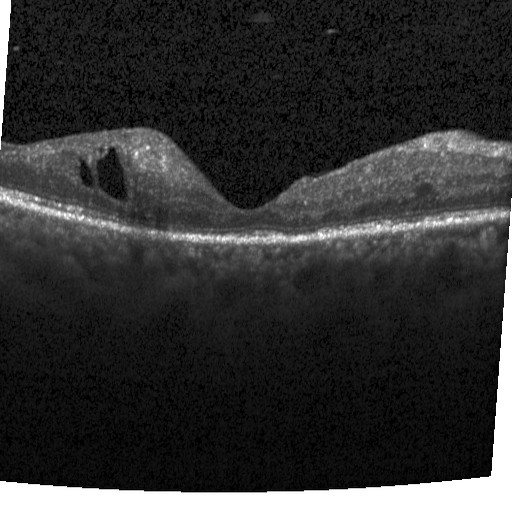

Retinal OCT B-scan — Diagnosis: diabetic macular edema.